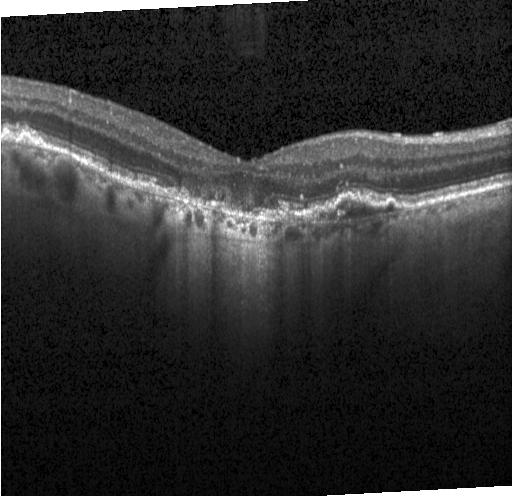 Dx: a choroidal neovascular membrane.